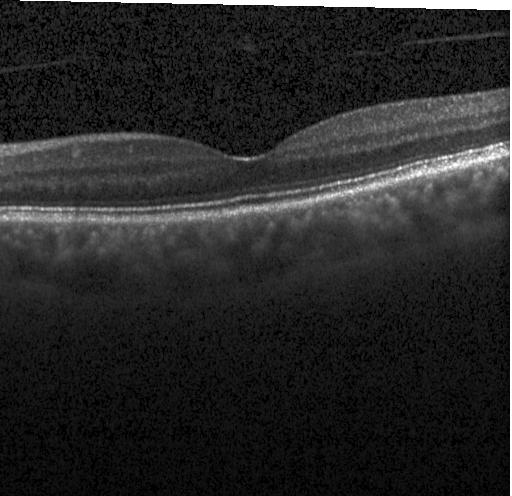
OCT line scan; spectral-domain optical coherence tomography; Heidelberg Spectralis
Finding: no CNV, no DME, and no drusen.